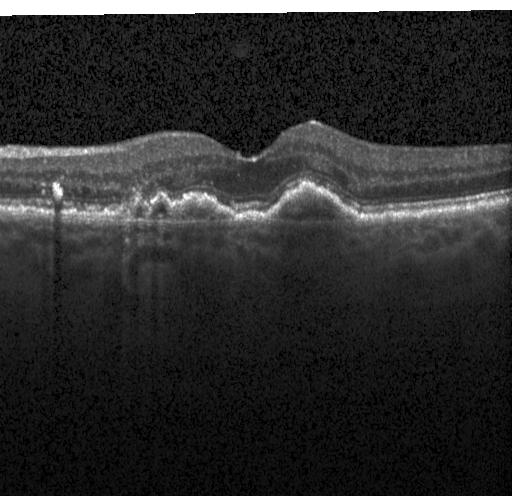

Impression: a choroidal neovascular membrane.